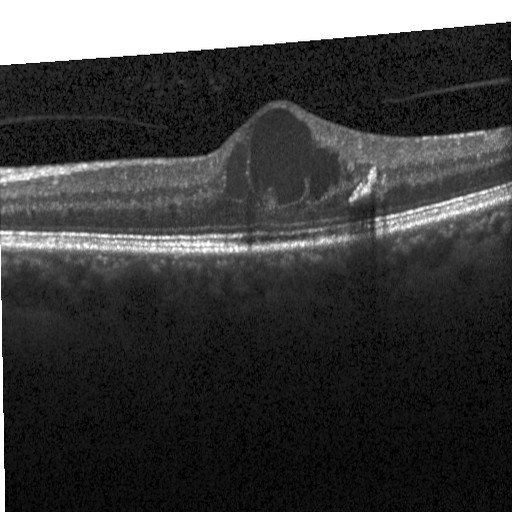

The scan shows diabetic macular edema.